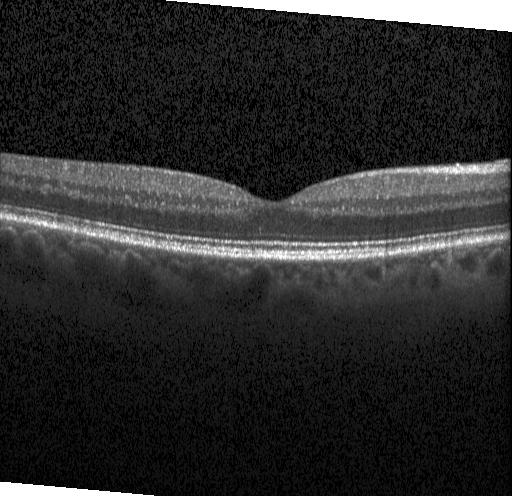 OCT scan showing no evidence of choroidal neovascularization, diabetic macular edema, or drusen.